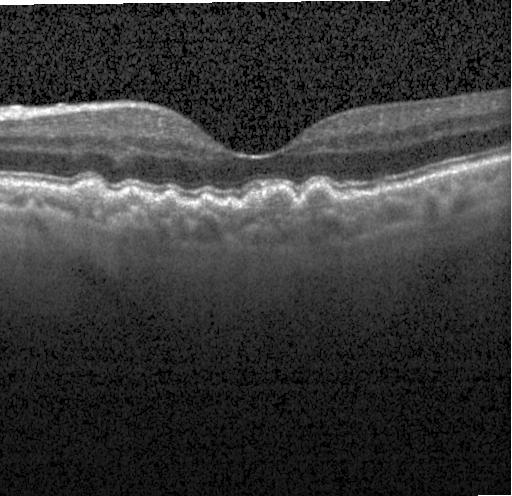

Retinal OCT B-scan. Assessment: sub-RPE drusenoid deposits.